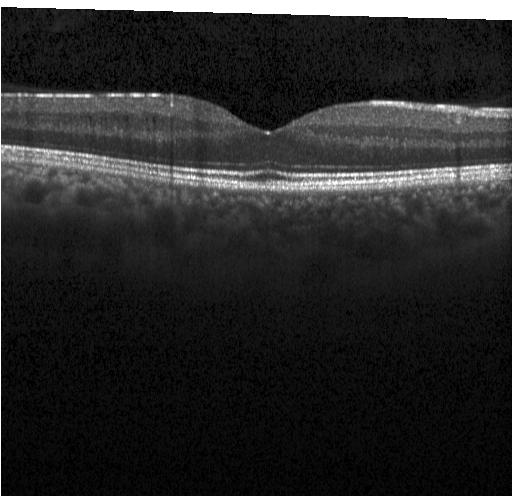

OCT B-scan
OCT finding: no choroidal neovascularization, diabetic macular edema, or drusen.